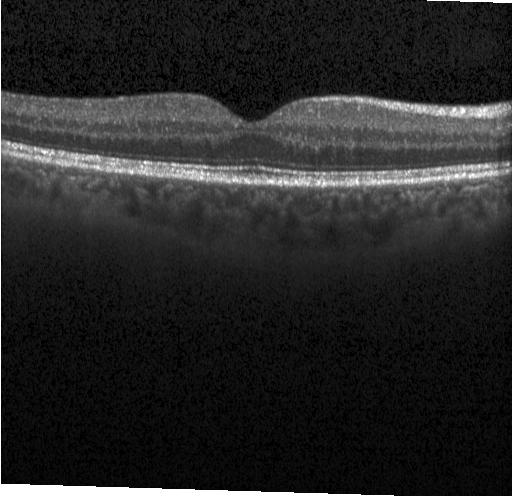 OCT finding: no evidence of choroidal neovascularization, diabetic macular edema, or drusen.